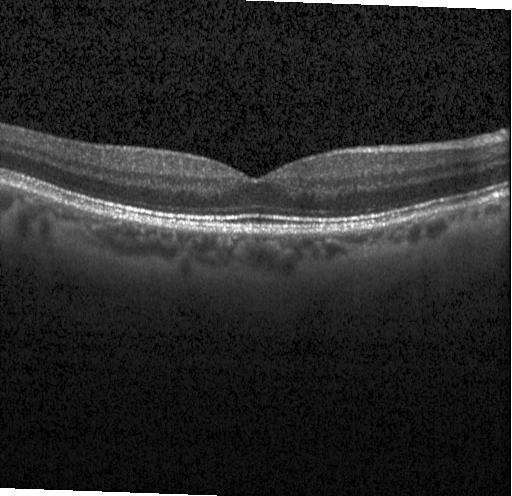

Through the macula. Optical coherence tomography scan
Dx: no CNV, DME, or drusen.